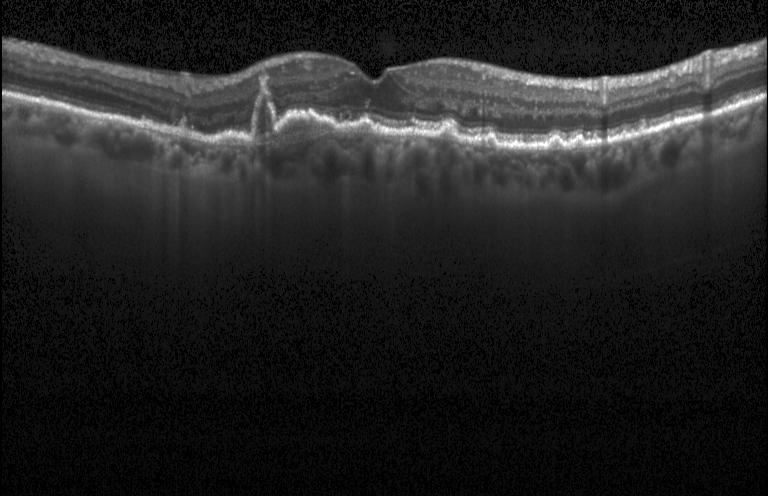
Optical coherence tomography B-scan. This B-scan demonstrates choroidal neovascularization (CNV).